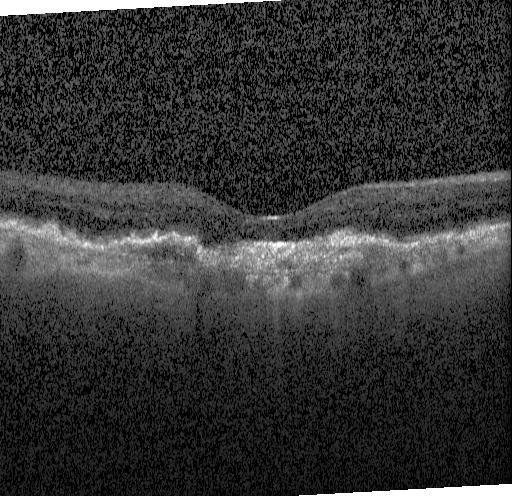 Centered on the fovea. OCT line scan. Spectral-domain OCT. Acquired on a Heidelberg Spectralis
Diagnosis: choroidal neovascularization.